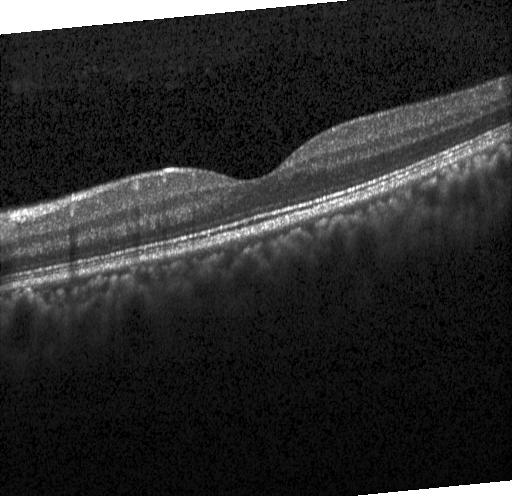
Spectral-domain optical coherence tomography; instrument: Heidelberg Spectralis; optical coherence tomography B-scan. Impression: neither CNV, DME, nor drusen.